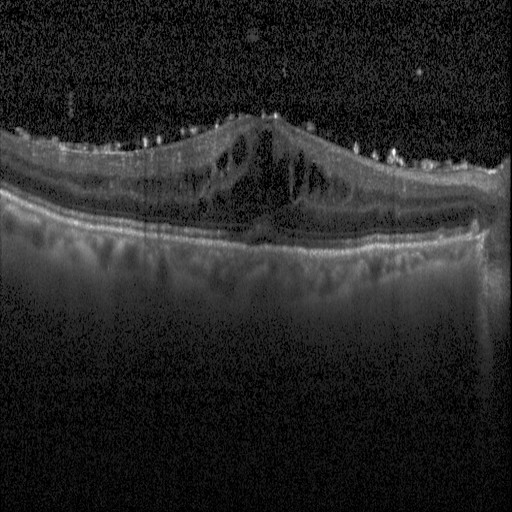
Diabetic macular edema.